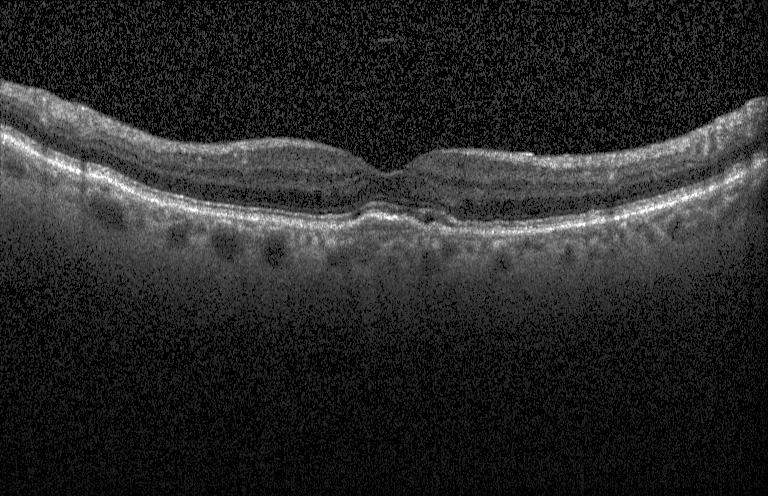

Choroidal neovascularization.